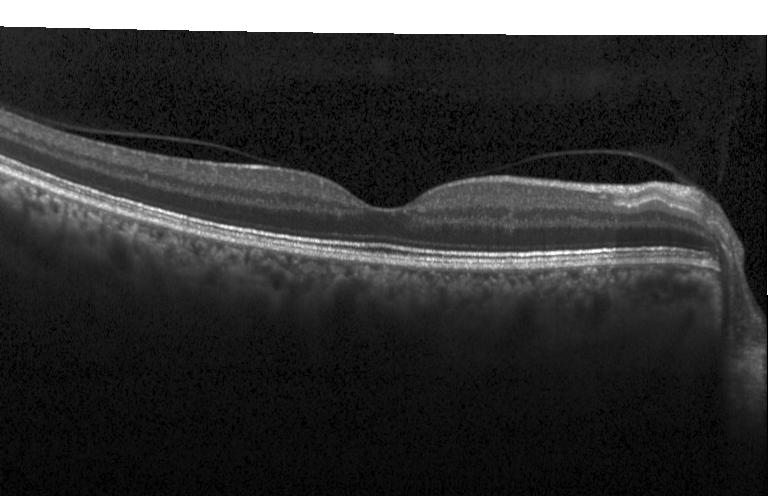

OCT B-scan · through the macula · instrument: Heidelberg Spectralis · SD-OCT
The scan shows neither choroidal neovascularization, diabetic macular edema, nor drusen.